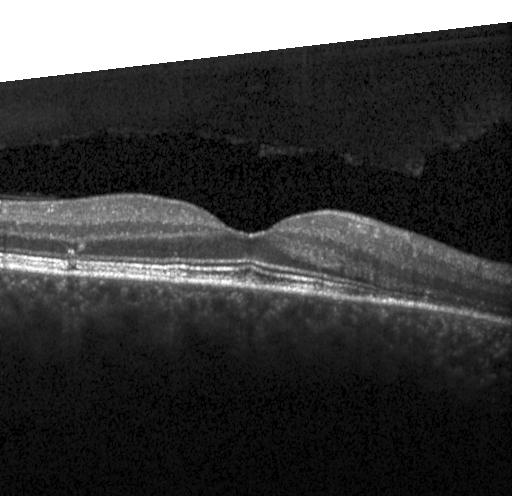 Retinal OCT cross-section
OCT finding: sub-RPE drusenoid deposits.